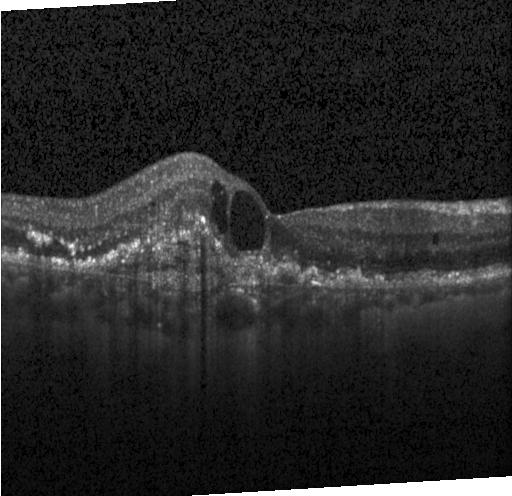 Retinal OCT cross-section, spectral-domain optical coherence tomography. The scan shows a choroidal neovascular membrane.